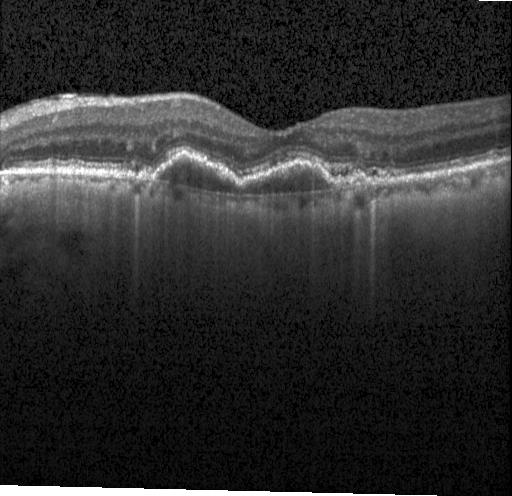
SD-OCT. Retinal OCT cross-section — Dx: CNV.